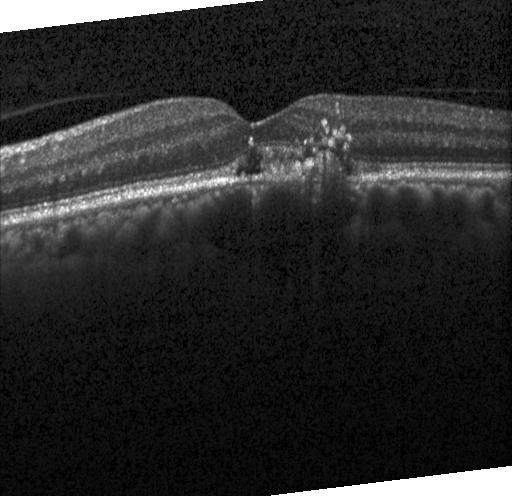

Heidelberg Spectralis, SD-OCT, through the macula, OCT line scan. Impression: a choroidal neovascular membrane.